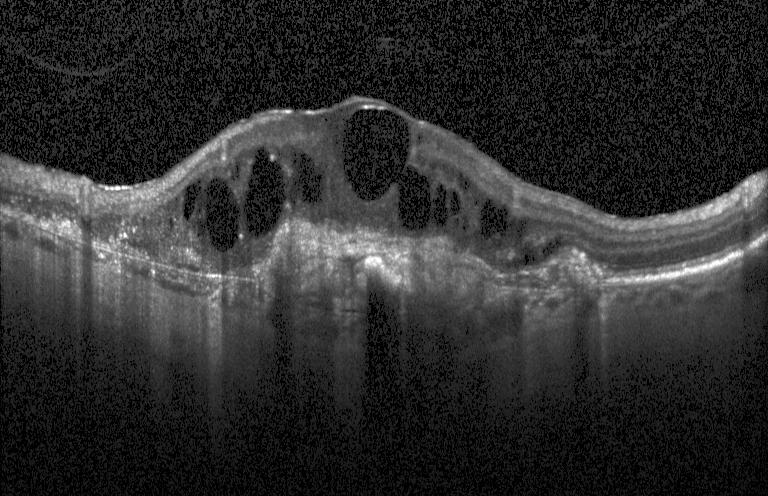
Spectral-domain OCT B-scan: a choroidal neovascular membrane.